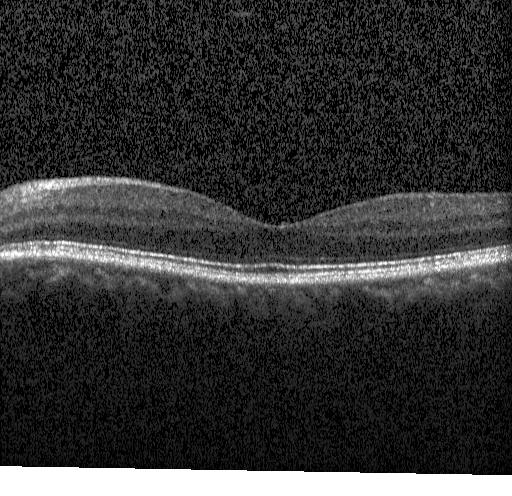
OCT line scan · instrument: Heidelberg Spectralis · spectral-domain OCT · horizontal scan through the fovea. Assessment: no CNV, DME, or drusen.